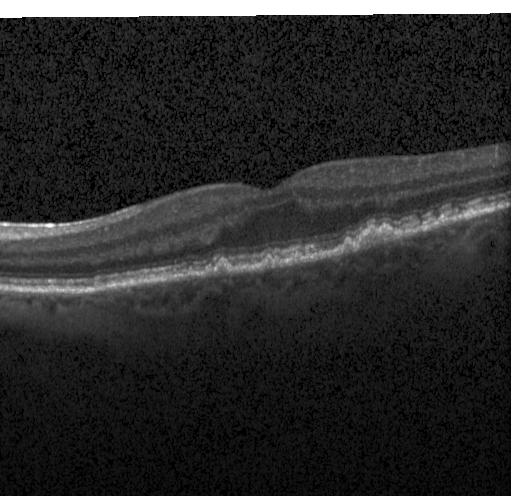 Diagnosis: sub-RPE drusenoid deposits.